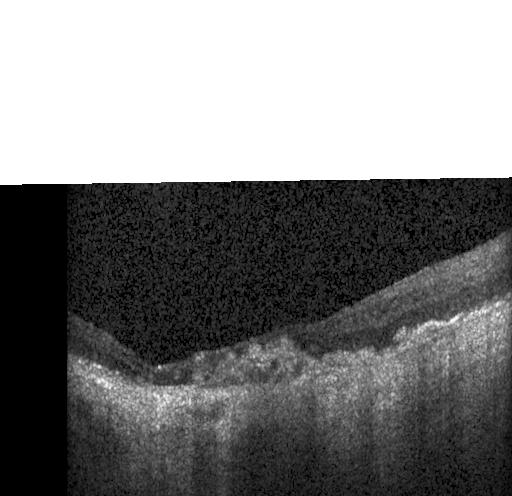

Instrument: Heidelberg Spectralis; fovea-centered; retinal OCT B-scan
Finding: choroidal neovascularization.